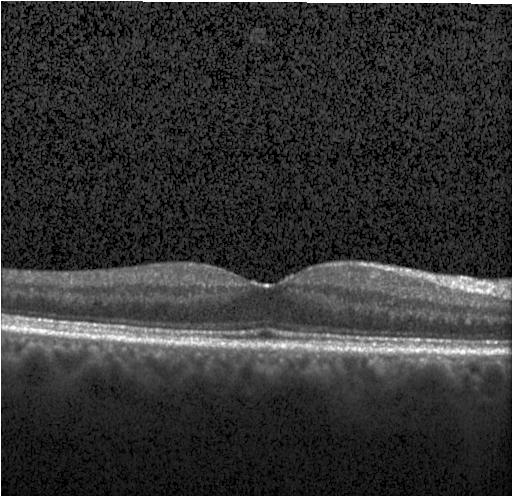 Dx: no choroidal neovascularization, diabetic macular edema, or drusen.